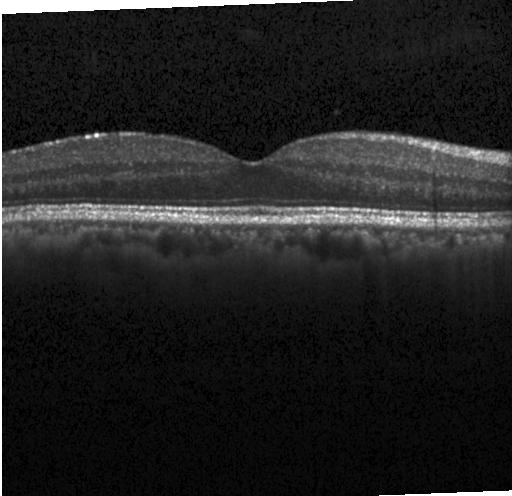

OCT B-scan, Heidelberg Spectralis, SD-OCT. OCT finding: no CNV, no DME, and no drusen.